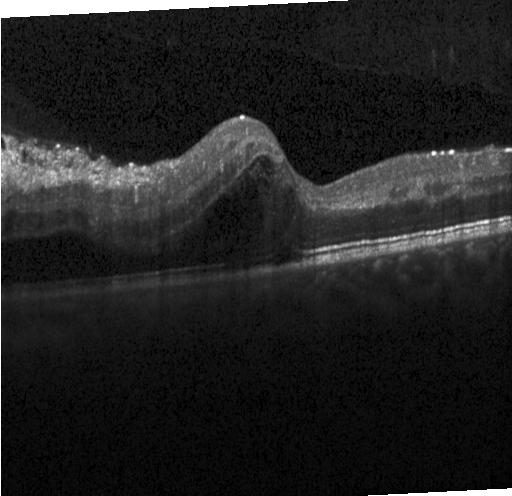
Optical coherence tomography B-scan. DME.